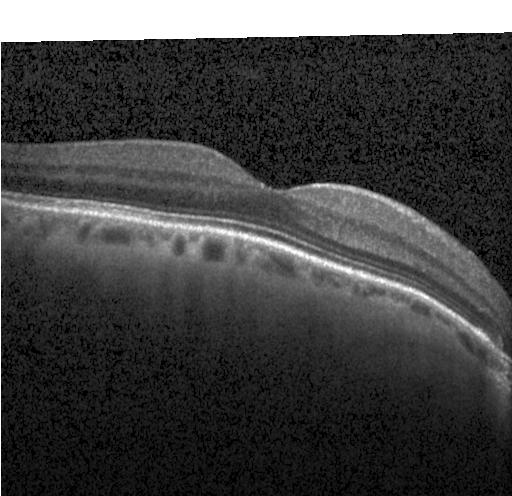

Macular OCT: no choroidal neovascularization, diabetic macular edema, or drusen.